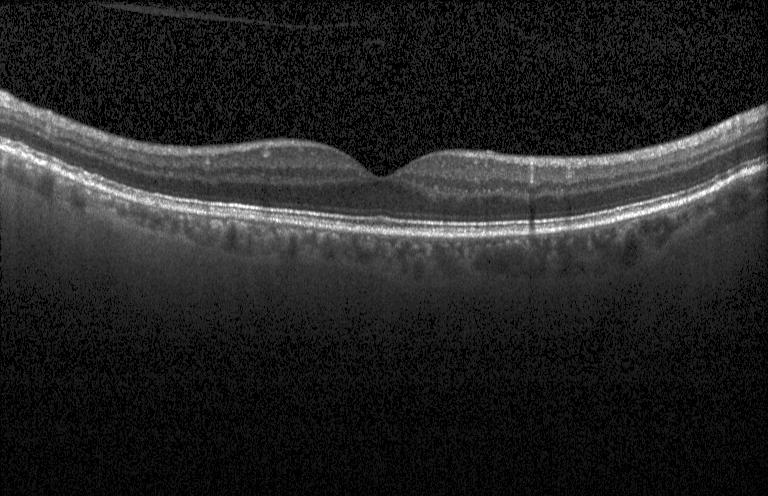
Horizontal scan through the fovea, retinal OCT B-scan, spectral-domain optical coherence tomography, acquired on a Heidelberg Spectralis — Diagnosis: no evidence of CNV, DME, or drusen.